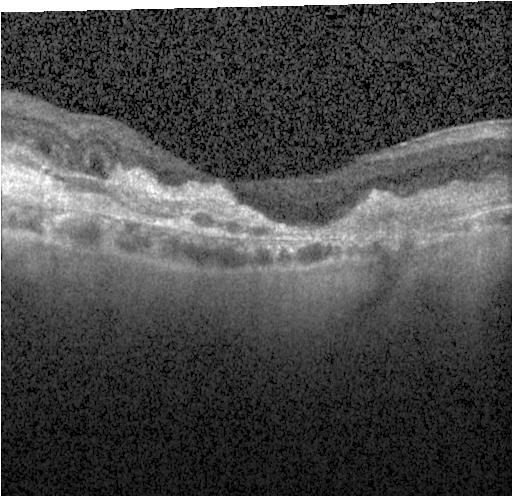

SD-OCT, acquired on a Heidelberg Spectralis, retinal OCT cross-section — Diagnosis: choroidal neovascularization.